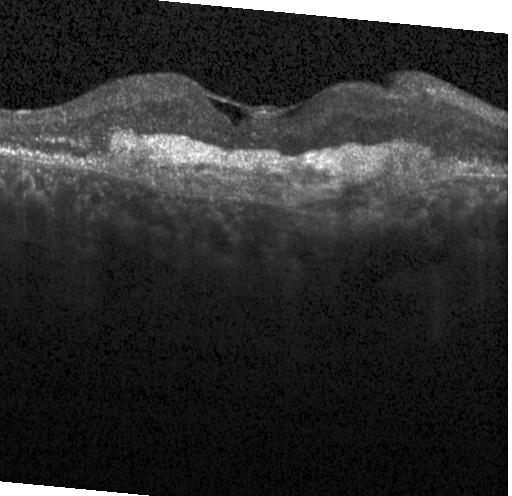 Macular OCT: a choroidal neovascular membrane.